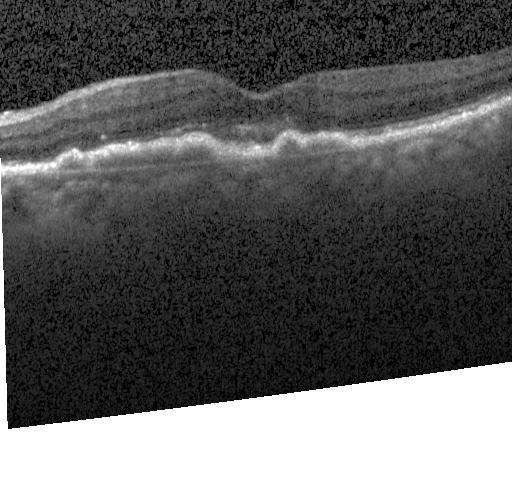 Assessment: choroidal neovascularization.